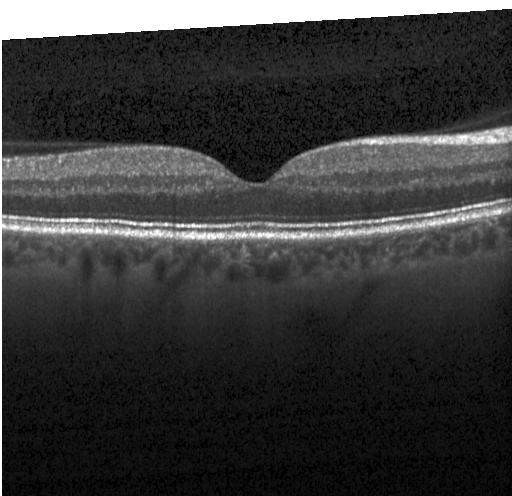

Retinal OCT cross-section
The scan shows no CNV, DME, or drusen.